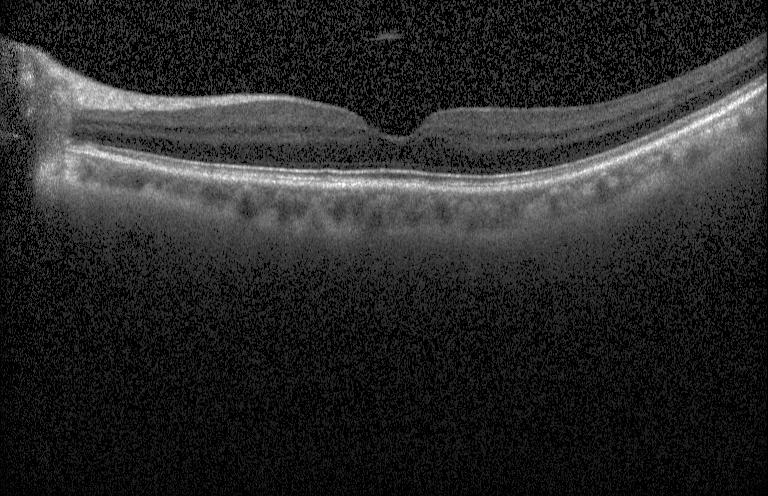 Optical coherence tomography B-scan, Heidelberg Spectralis, macular scan — No evidence of CNV, DME, or drusen.